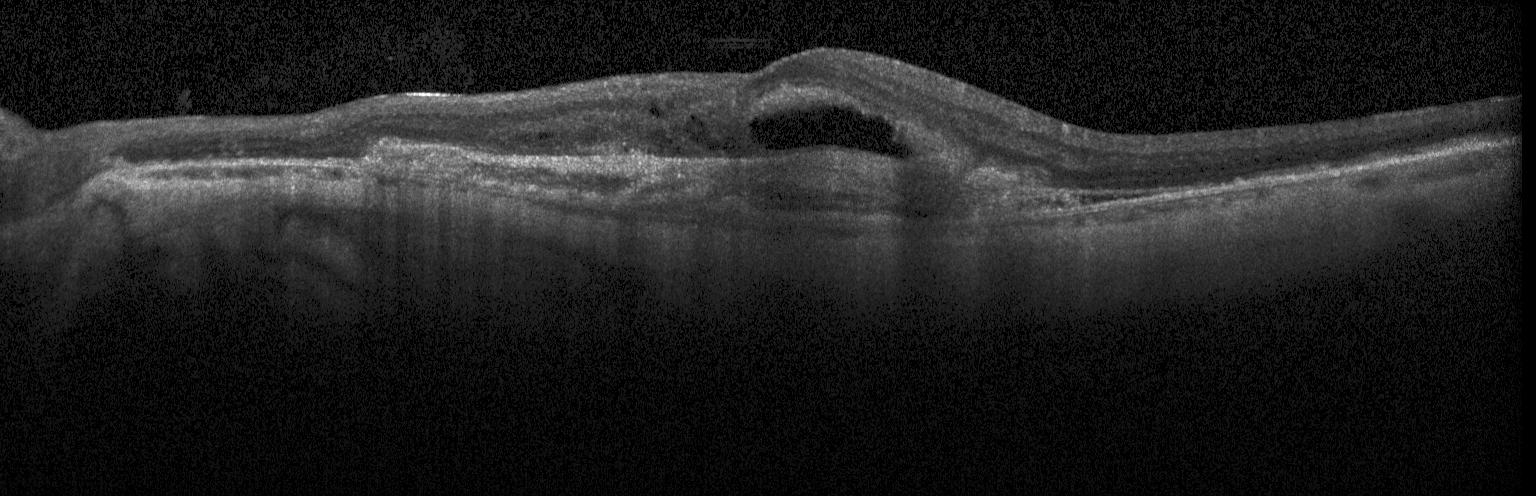
Impression: a choroidal neovascular membrane.